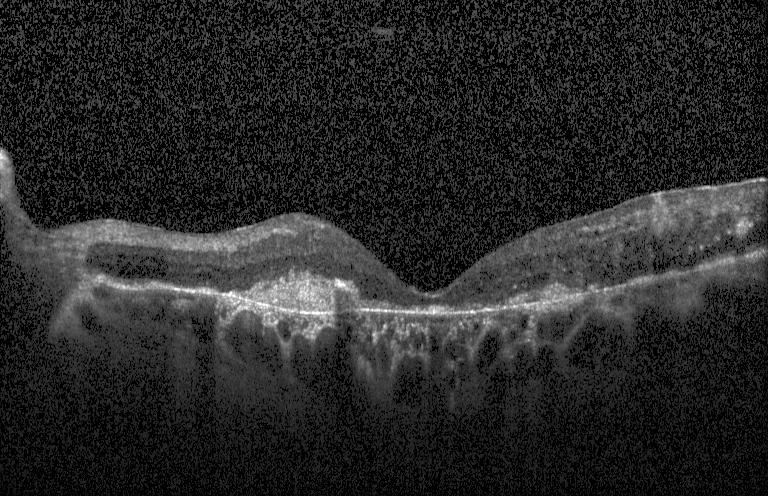 Heidelberg Spectralis OCT system; fovea-centered; optical coherence tomography B-scan. Impression: a choroidal neovascular membrane.